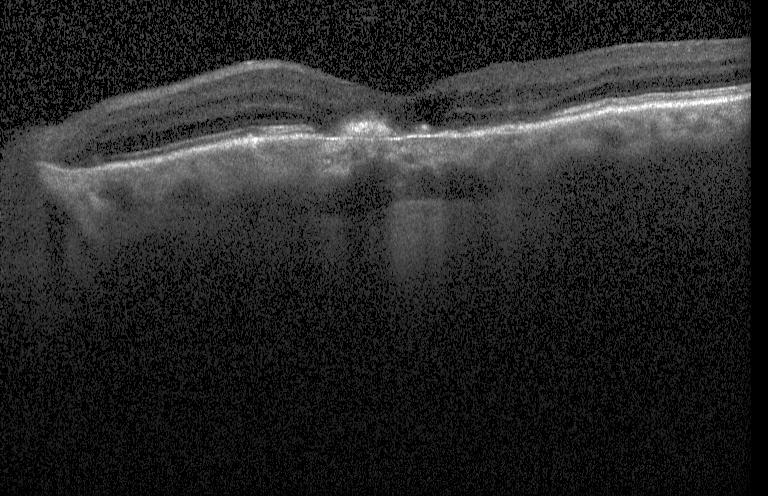 OCT B-scan — Assessment: choroidal neovascularization.